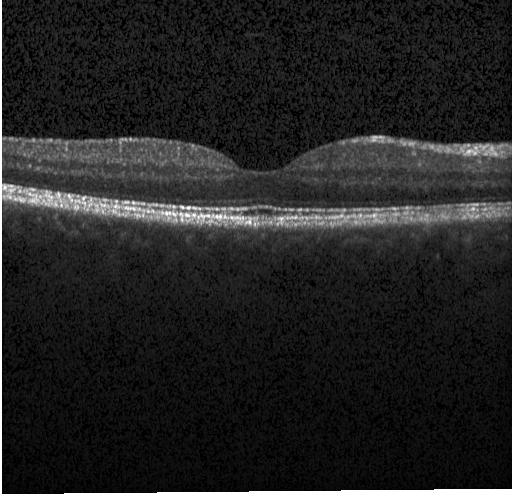
Heidelberg Spectralis · horizontal scan through the fovea · spectral-domain optical coherence tomography · OCT line scan.
OCT finding: no choroidal neovascularization, diabetic macular edema, or drusen.